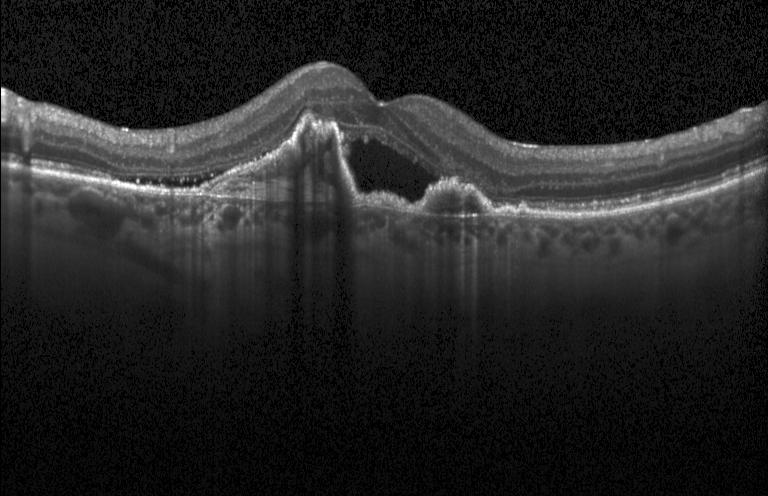

Spectral-domain OCT B-scan: a choroidal neovascular membrane.